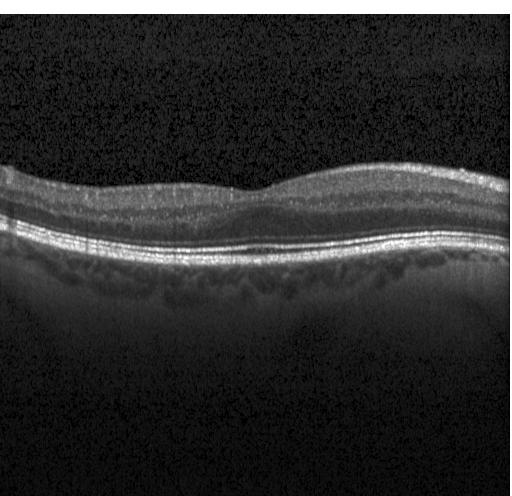 OCT line scan. Diagnosis: no evidence of CNV, DME, or drusen.